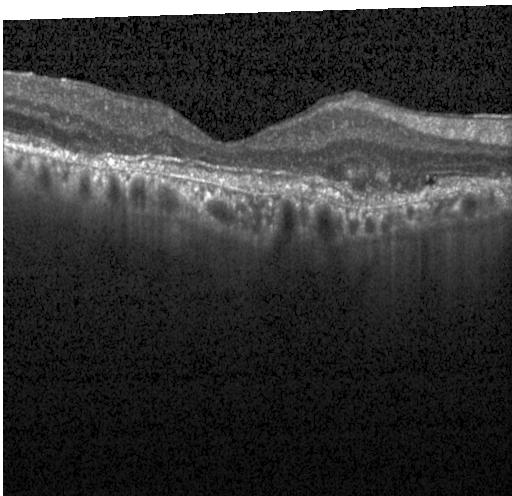 Impression: a choroidal neovascular membrane.